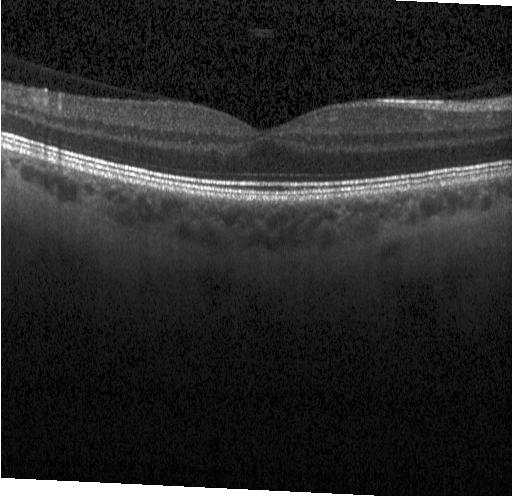
Finding: no choroidal neovascularization, no diabetic macular edema, and no drusen.